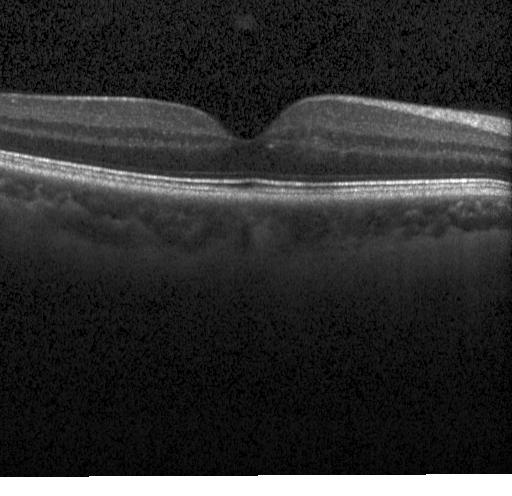

Diagnosis: no evidence of choroidal neovascularization, diabetic macular edema, or drusen.